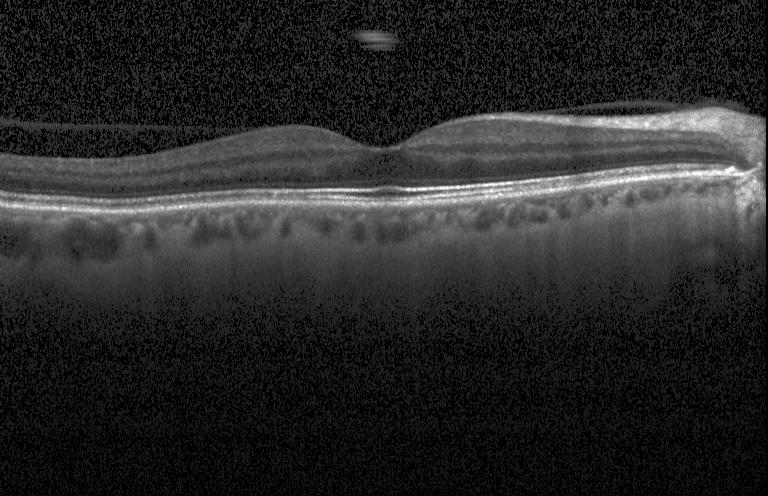 Optical coherence tomography B-scan, instrument: Heidelberg Spectralis, spectral-domain OCT. Impression: no choroidal neovascularization, no diabetic macular edema, and no drusen.